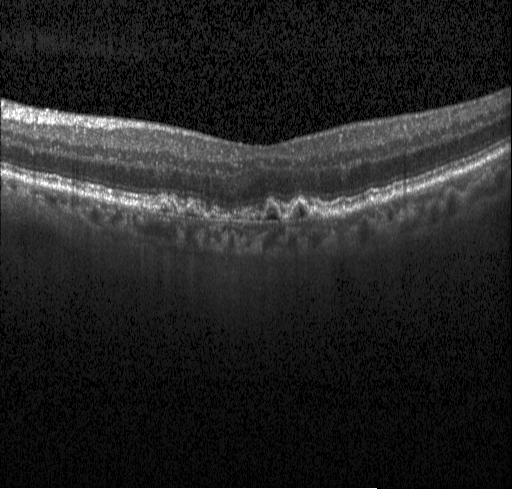

Dx: drusen.